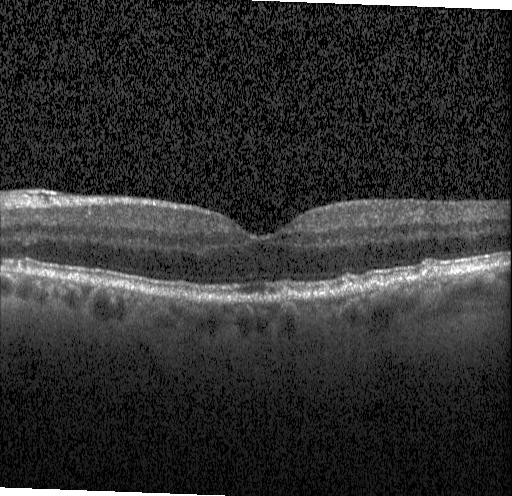

Diagnosis: sub-RPE drusenoid deposits.